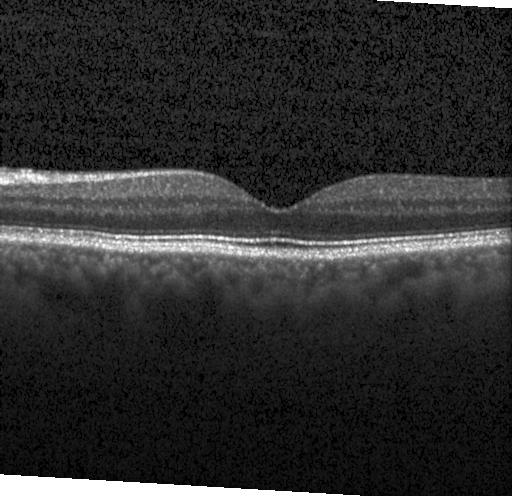 Retinal OCT B-scan — Diagnosis: no CNV, DME, or drusen.